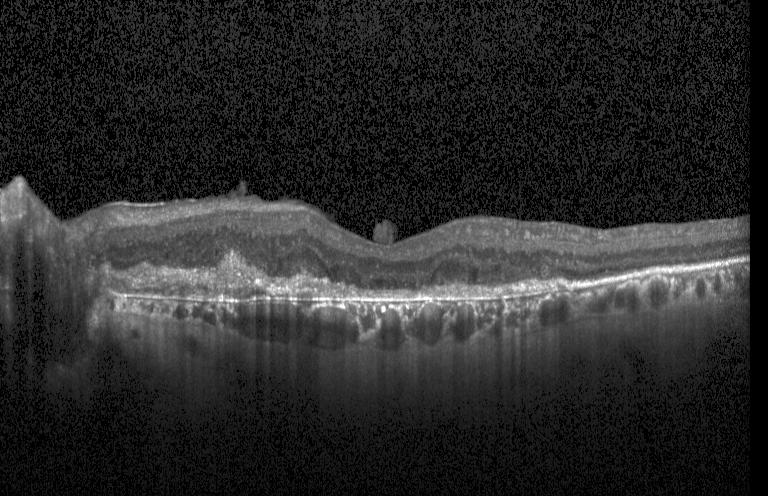
OCT B-scan showing choroidal neovascularization (CNV).